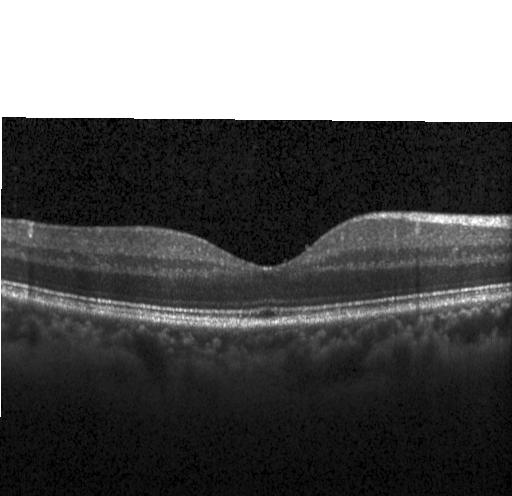
Retinal OCT cross-section
Finding: neither choroidal neovascularization, diabetic macular edema, nor drusen.